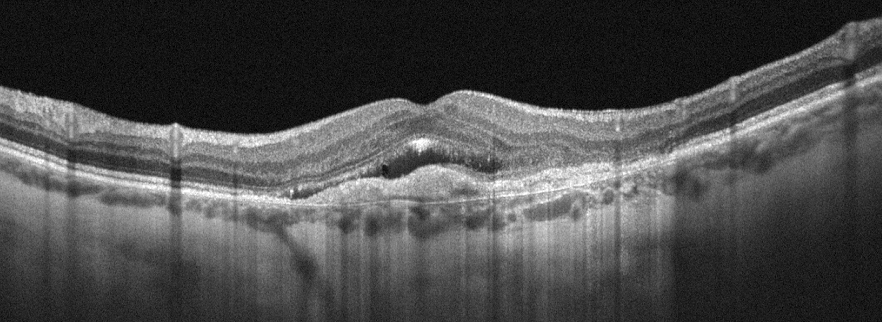 Optical coherence tomography scan, OD — Assessment: age-related macular degeneration (AMD).